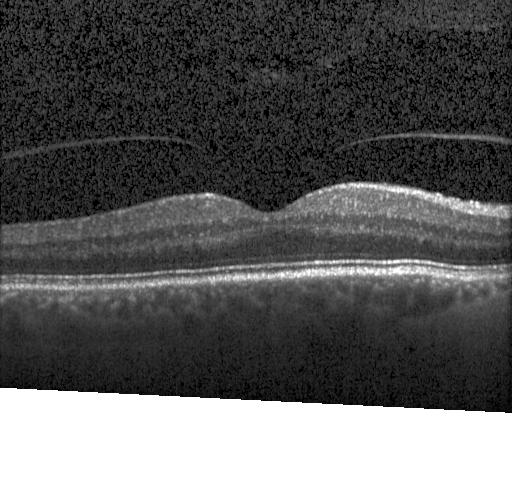
Acquired on a Heidelberg Spectralis · optical coherence tomography B-scan · through the macula
Diagnosis: neither CNV, DME, nor drusen.